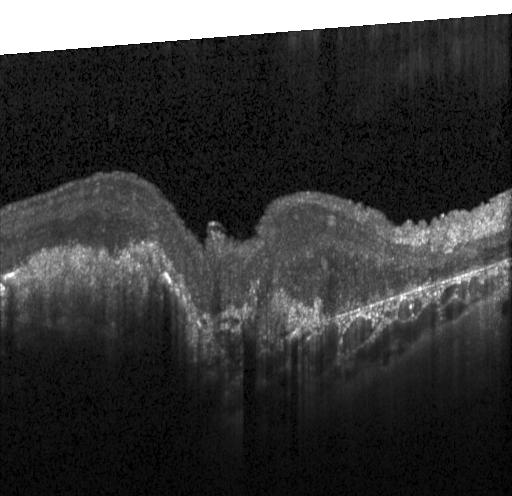 This B-scan demonstrates CNV.